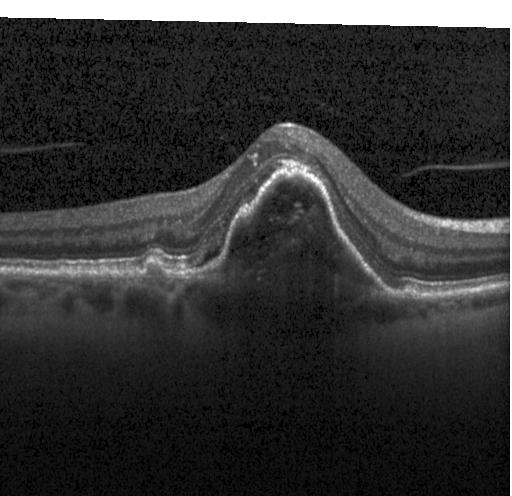 Macular scan. Optical coherence tomography scan. This B-scan demonstrates CNV.